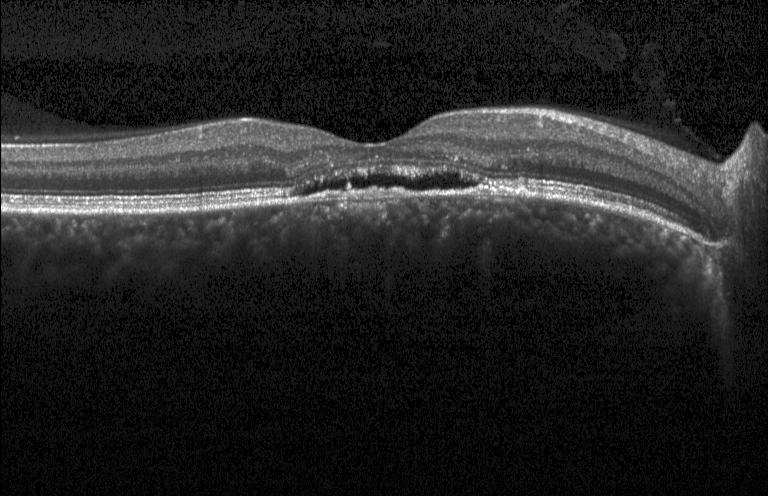 Heidelberg Spectralis. OCT line scan. Dx: a choroidal neovascular membrane.